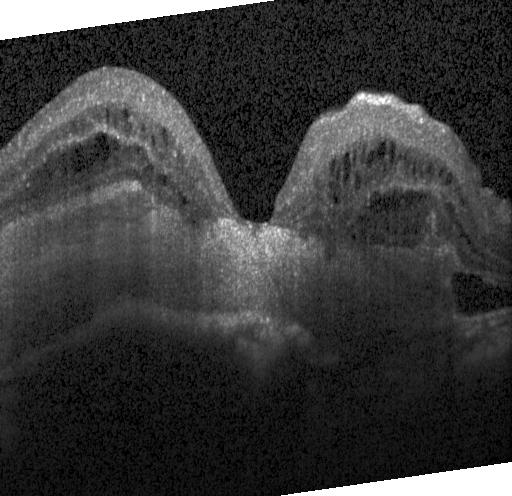
Instrument: Heidelberg Spectralis. Optical coherence tomography B-scan. Through the macula. SD-OCT
Assessment: a choroidal neovascular membrane.